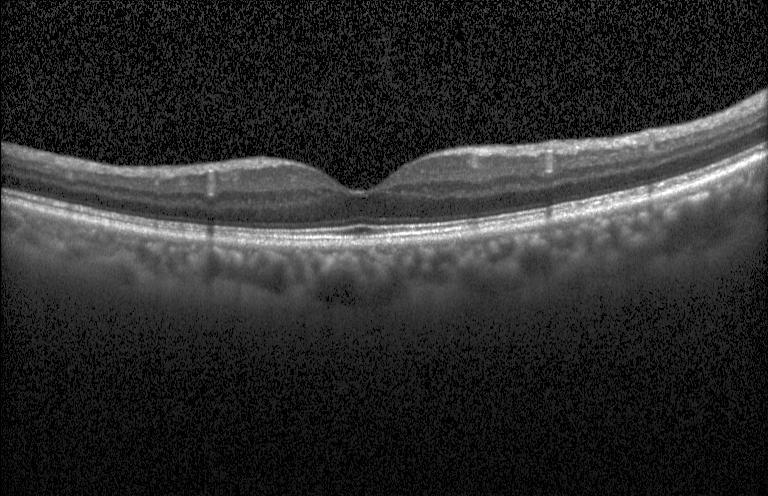

Retinal OCT cross-section — Diagnosis: no evidence of CNV, DME, or drusen.